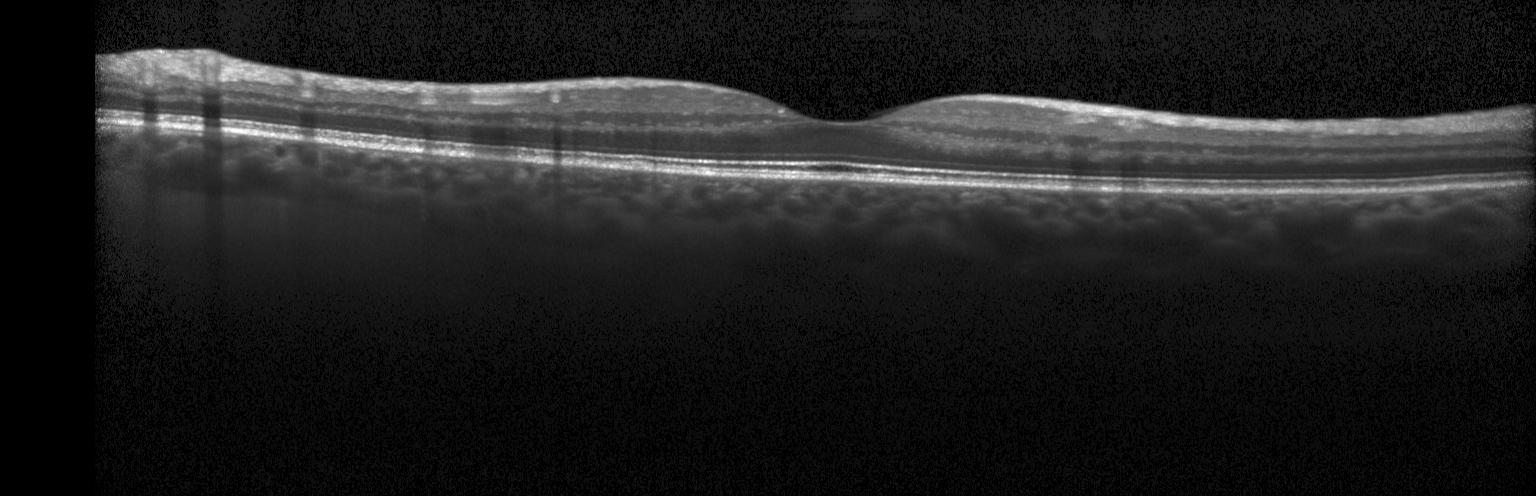
OCT scan showing no CNV, no DME, and no drusen.